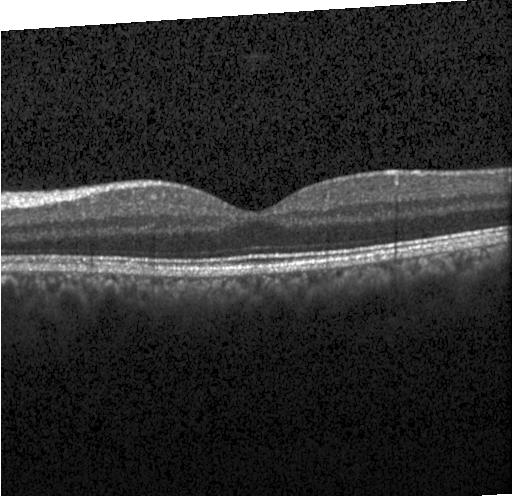 The scan shows neither CNV, DME, nor drusen.